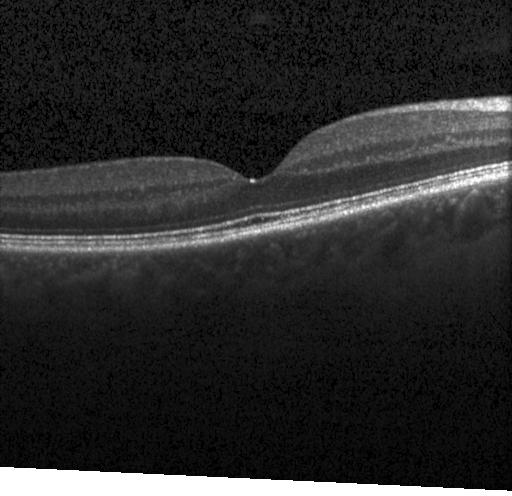
Macular OCT: no evidence of choroidal neovascularization, diabetic macular edema, or drusen.